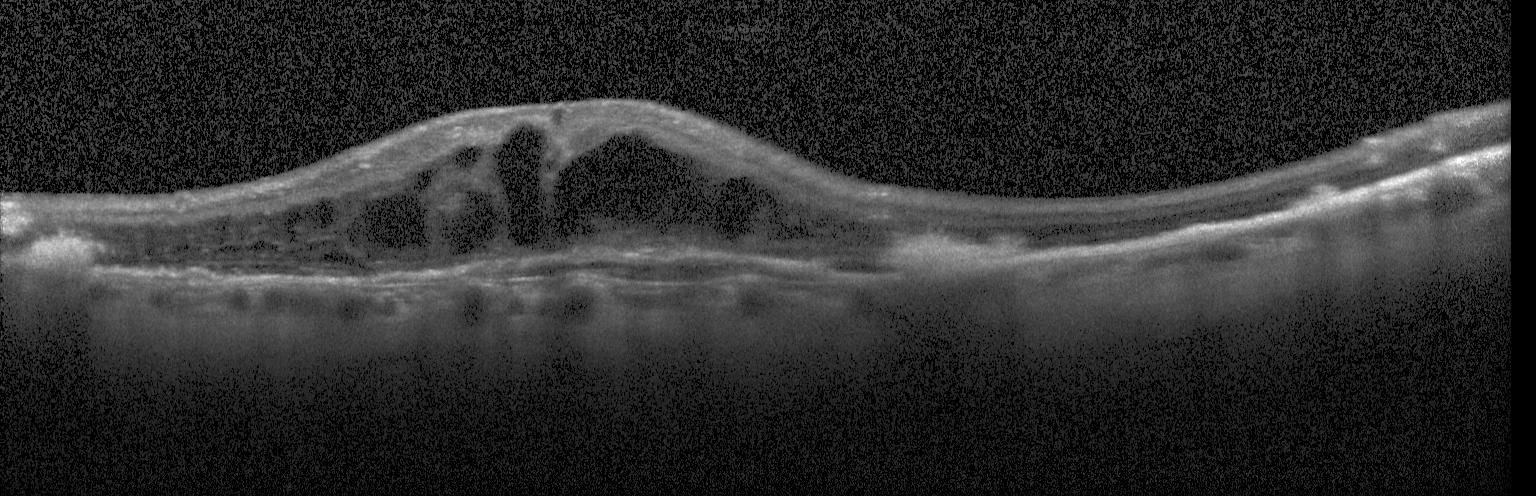 Retinal OCT B-scan — Assessment: choroidal neovascularization.